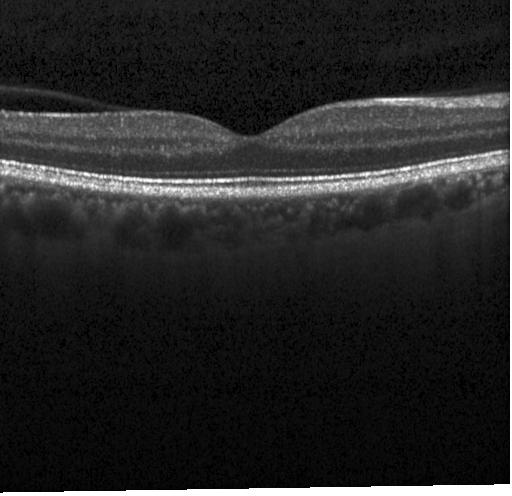 Retinal OCT cross-section. Diagnosis: no CNV, no DME, and no drusen.